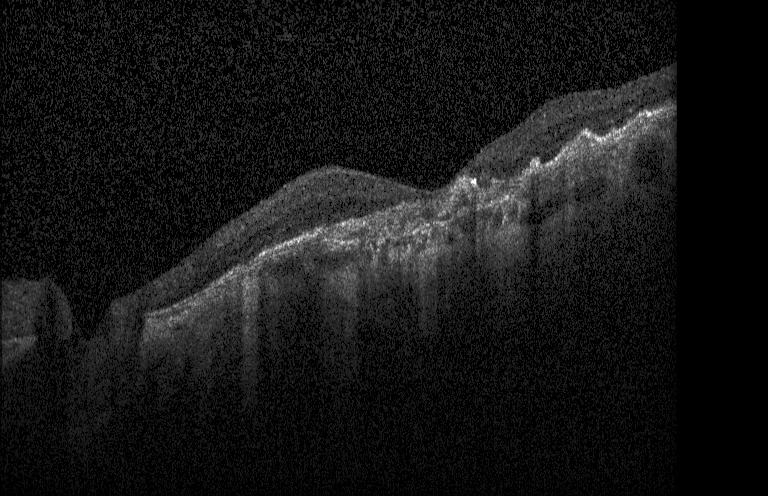 Spectral-domain OCT · OCT line scan · Heidelberg Spectralis OCT system — Dx: CNV.